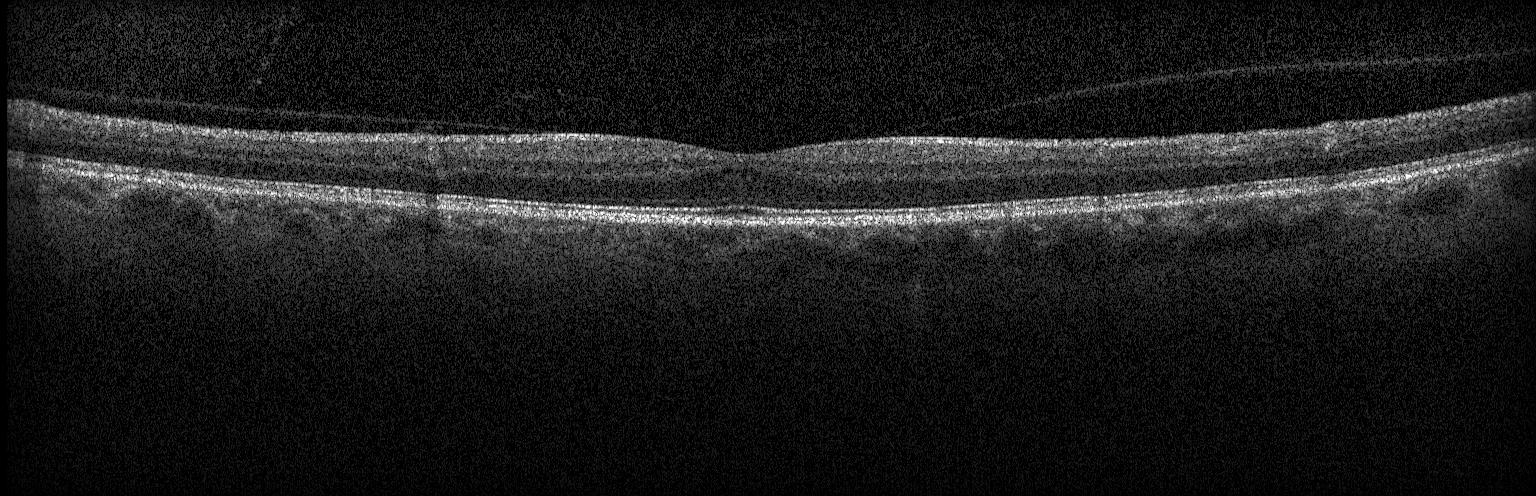
Heidelberg Spectralis · optical coherence tomography scan · spectral-domain OCT · horizontal scan through the fovea
This B-scan demonstrates no choroidal neovascularization, no diabetic macular edema, and no drusen.